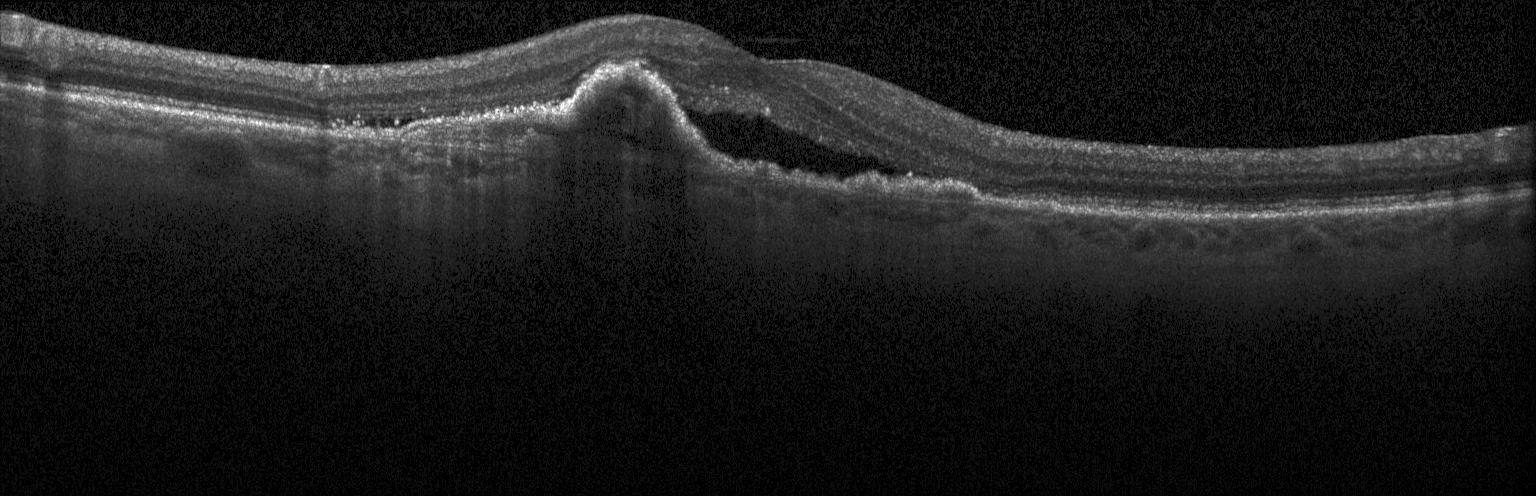

Spectral-domain OCT, through the macula, optical coherence tomography B-scan, Heidelberg Spectralis
Dx: a choroidal neovascular membrane.